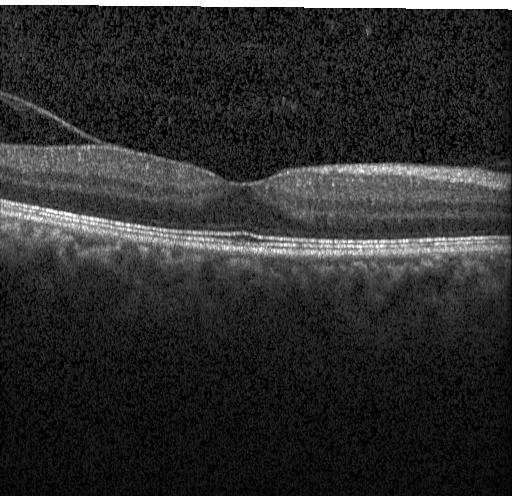
Retinal OCT cross-section.
Assessment: no CNV, DME, or drusen.